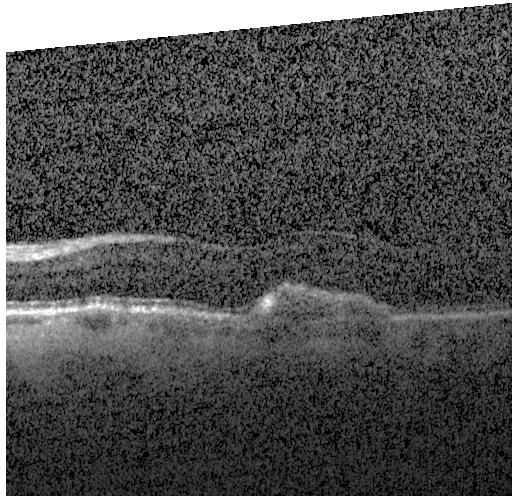

Optical coherence tomography scan.
Finding: choroidal neovascularization.